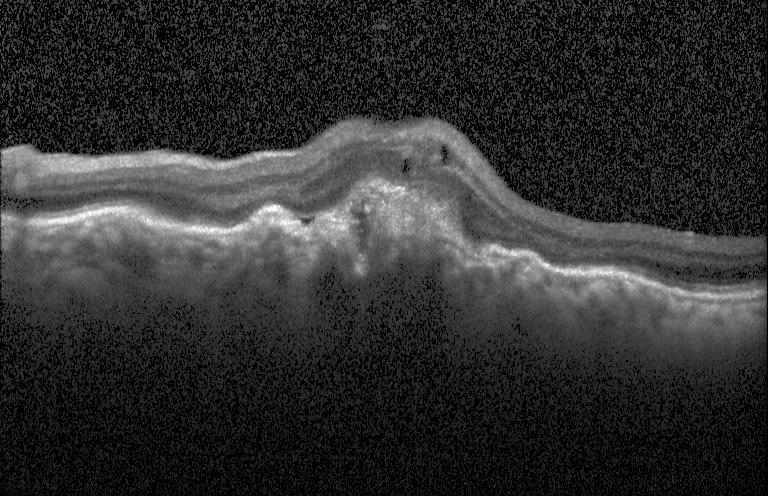
Retinal OCT cross-section.
Diagnosis: a choroidal neovascular membrane.